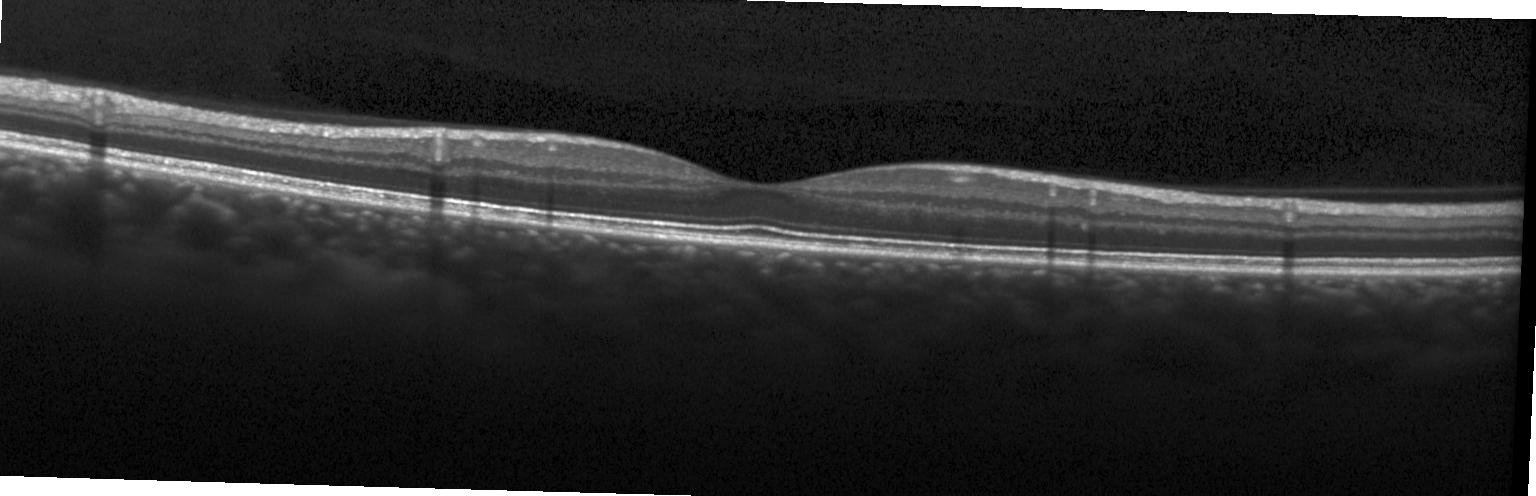 Retinal OCT B-scan, centered on the fovea
Assessment: no choroidal neovascularization, no diabetic macular edema, and no drusen.